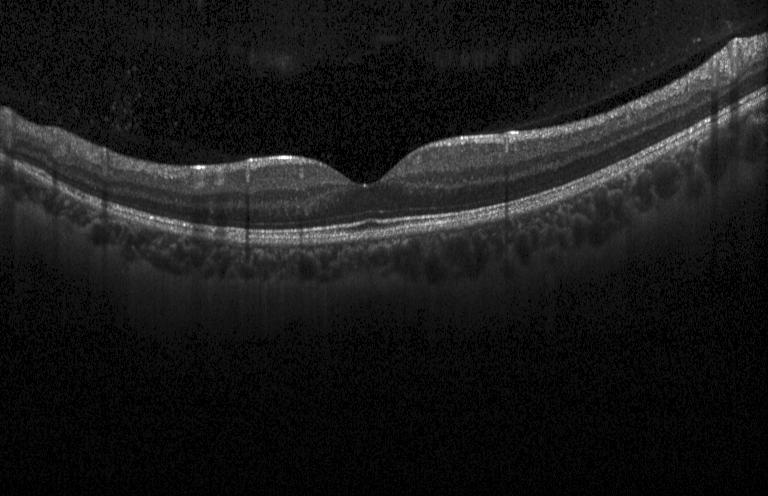 Fovea-centered · SD-OCT · OCT B-scan — The scan shows neither choroidal neovascularization, diabetic macular edema, nor drusen.